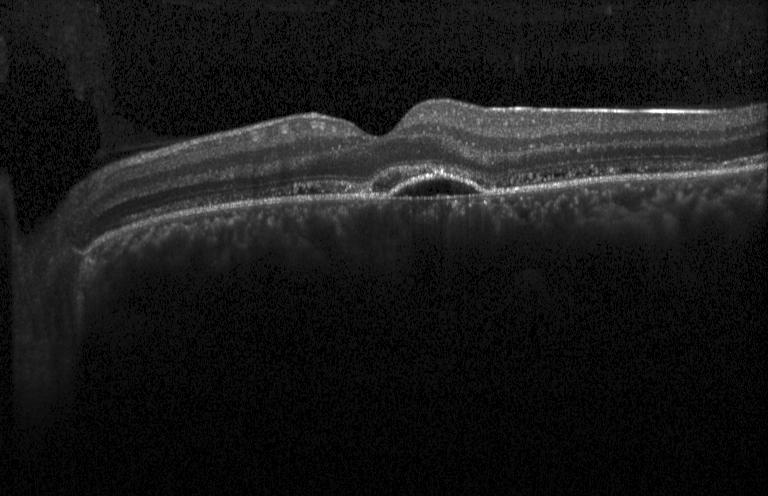
Heidelberg Spectralis OCT system; retinal OCT cross-section
Assessment: a choroidal neovascular membrane.